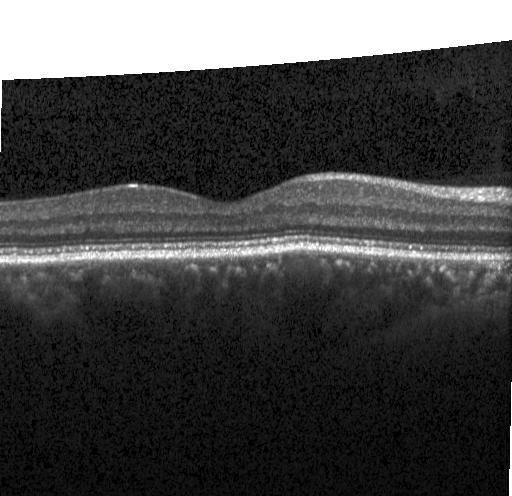

Acquired on a Heidelberg Spectralis · retinal OCT B-scan · SD-OCT · horizontal scan through the fovea. Neither choroidal neovascularization, diabetic macular edema, nor drusen.